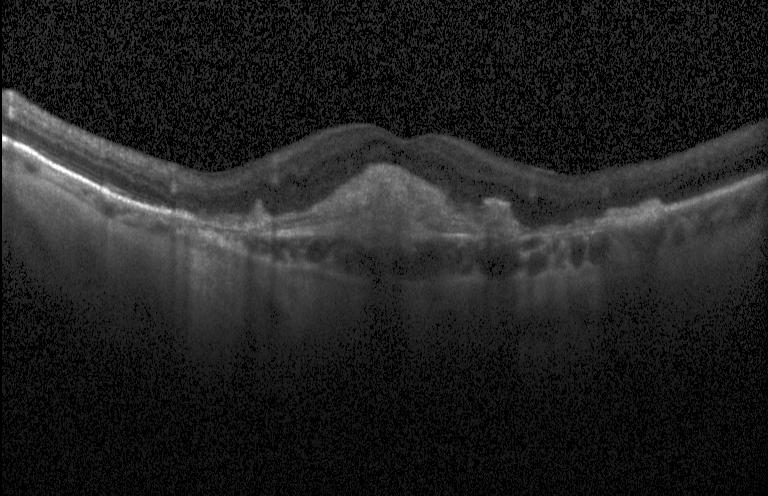
OCT finding: choroidal neovascularization.